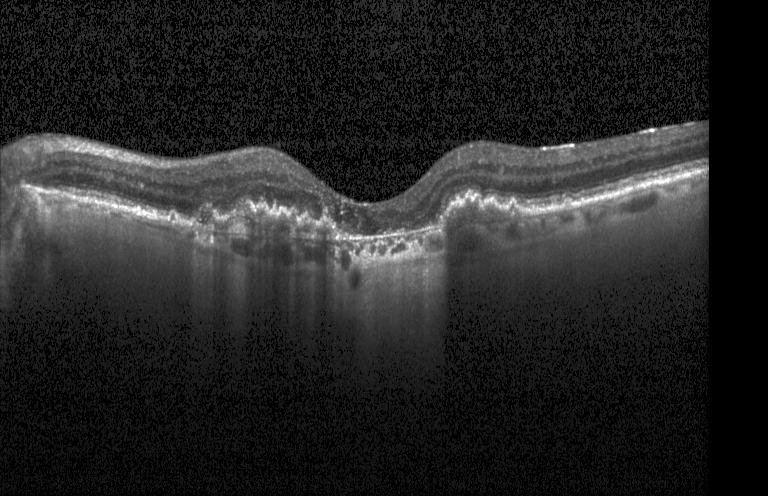
Optical coherence tomography B-scan · through the macula · SD-OCT · Heidelberg Spectralis OCT system. Diagnosis: CNV.